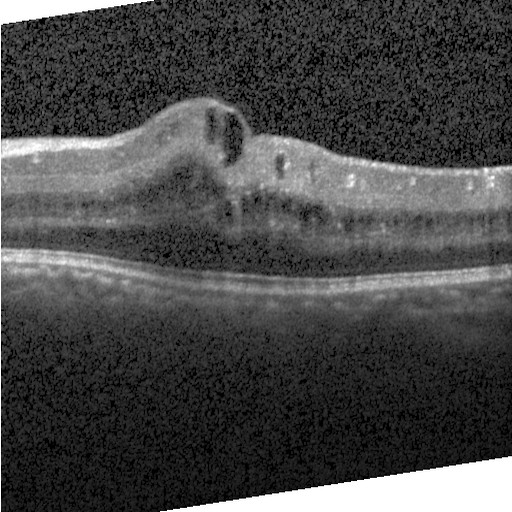 OCT line scan.
Diagnosis: DME.